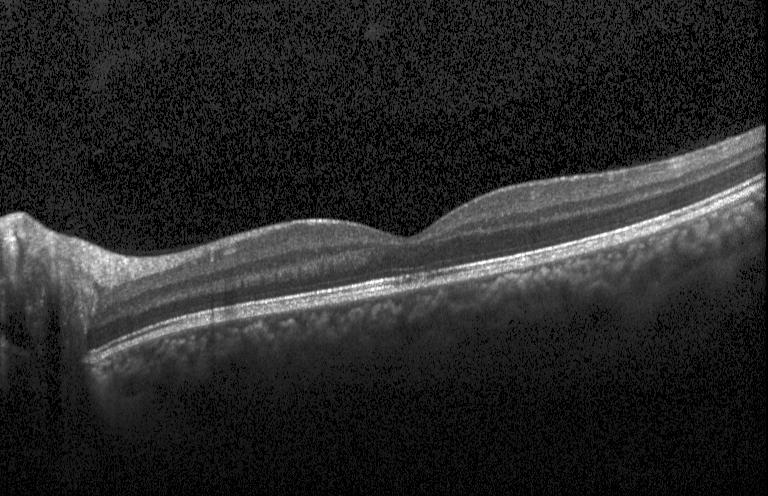

Retinal OCT cross-section; instrument: Heidelberg Spectralis; through the macula.
Assessment: neither CNV, DME, nor drusen.